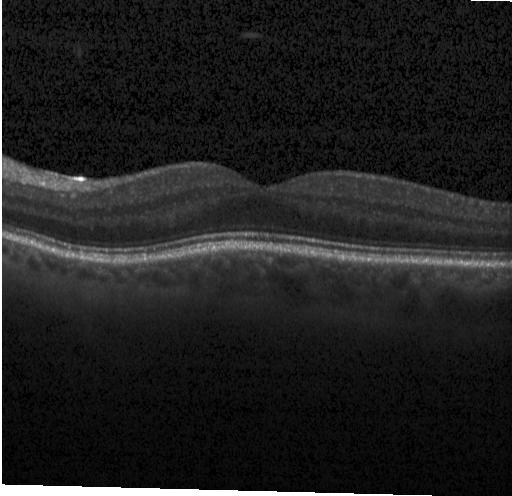 Retinal OCT B-scan.
Diagnosis: no choroidal neovascularization, diabetic macular edema, or drusen.